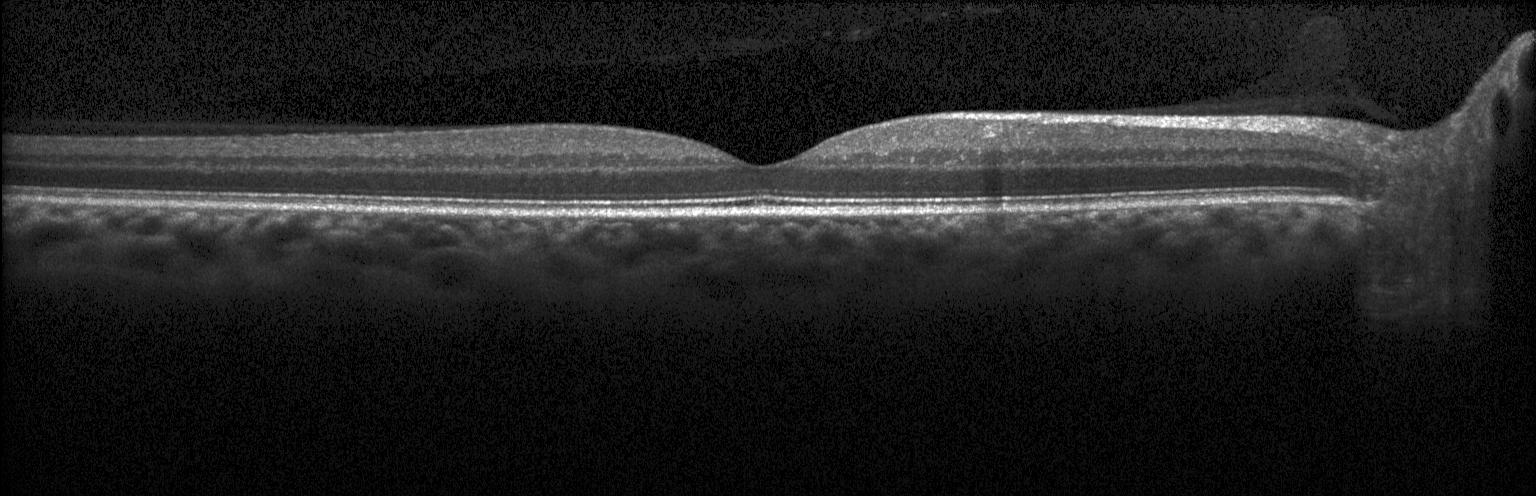

Retinal OCT B-scan · through the macula · Heidelberg Spectralis.
Assessment: no CNV, no DME, and no drusen.